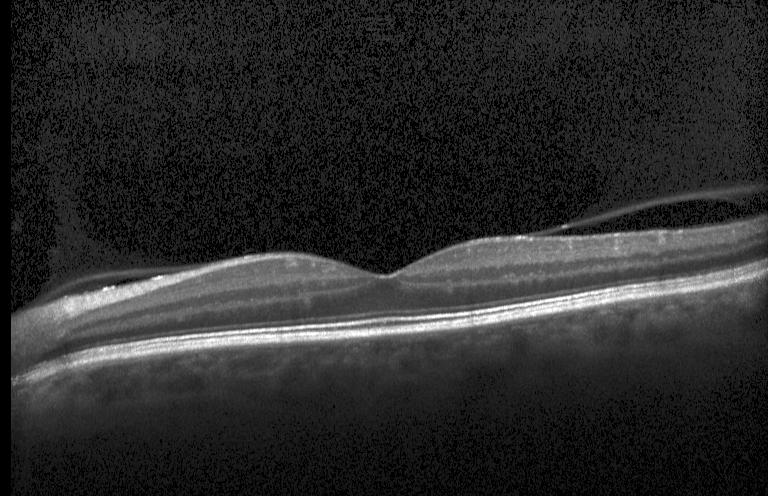 OCT B-scan
Assessment: no choroidal neovascularization, diabetic macular edema, or drusen.